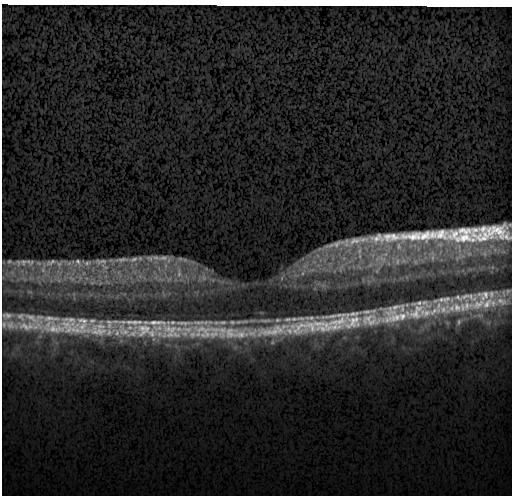
Optical coherence tomography scan.
Macular OCT: no CNV, no DME, and no drusen.